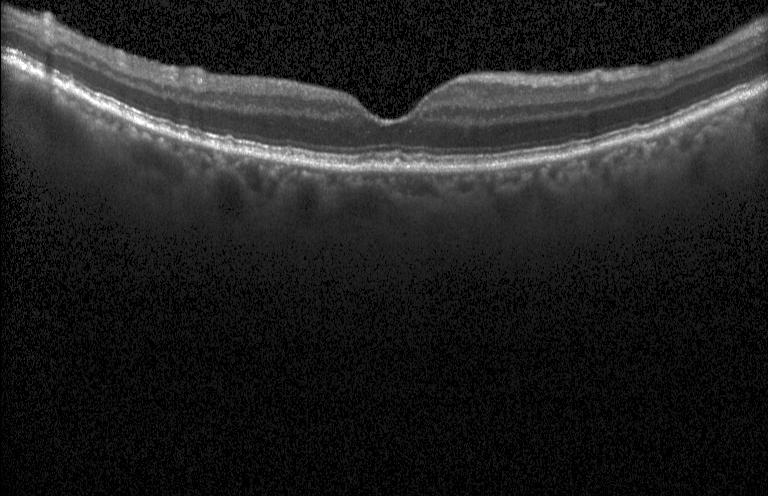 Diagnosis: multiple drusen.